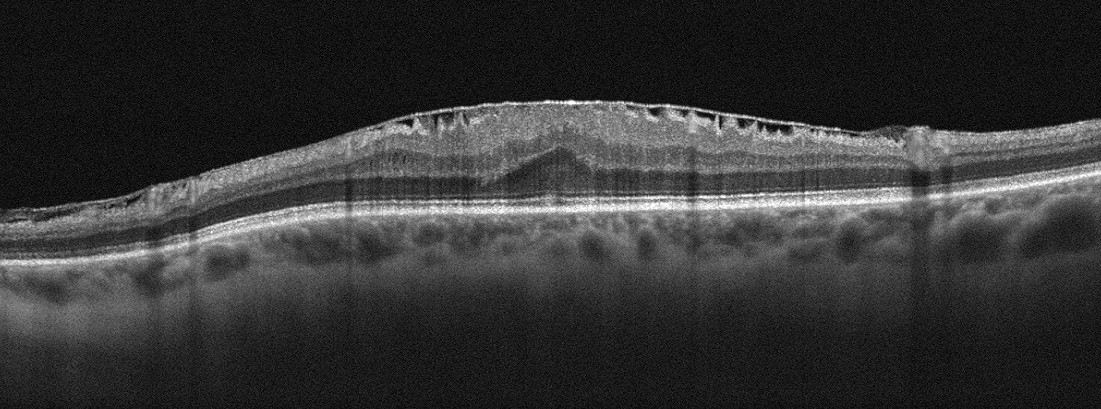

Retinal OCT cross-section showing epiretinal membrane.